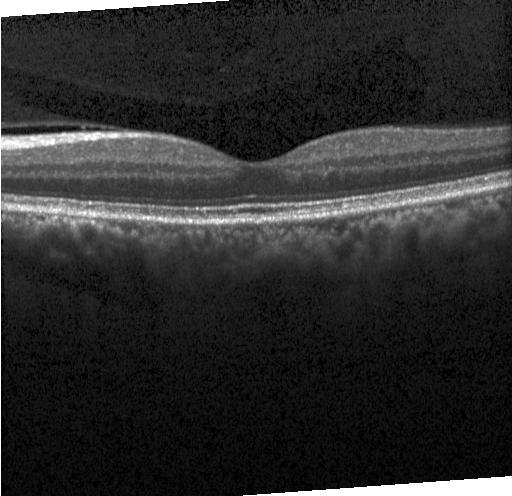 Dx: no choroidal neovascularization, no diabetic macular edema, and no drusen.